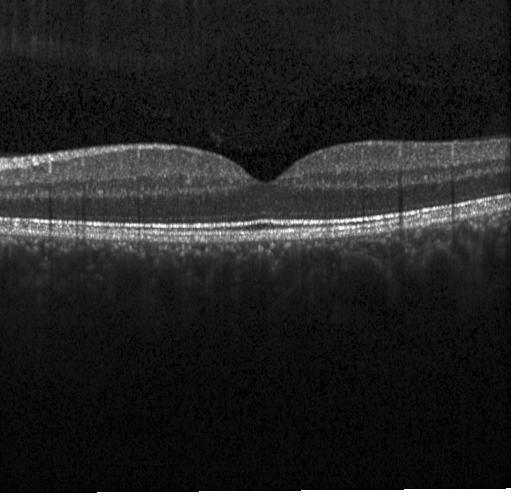
Horizontal scan through the fovea; optical coherence tomography B-scan; spectral-domain OCT; Heidelberg Spectralis OCT system — Diagnosis: no choroidal neovascularization, no diabetic macular edema, and no drusen.